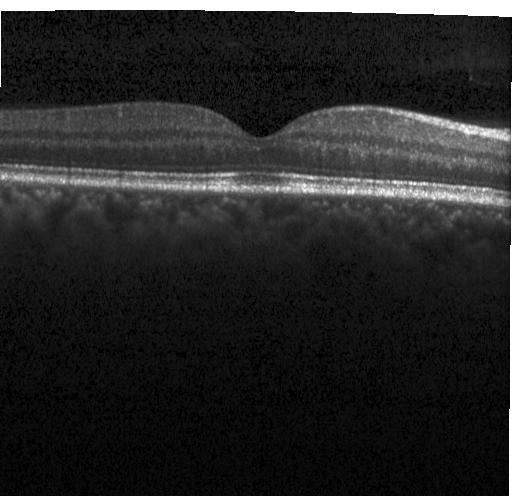
SD-OCT; optical coherence tomography B-scan
Impression: no CNV, no DME, and no drusen.